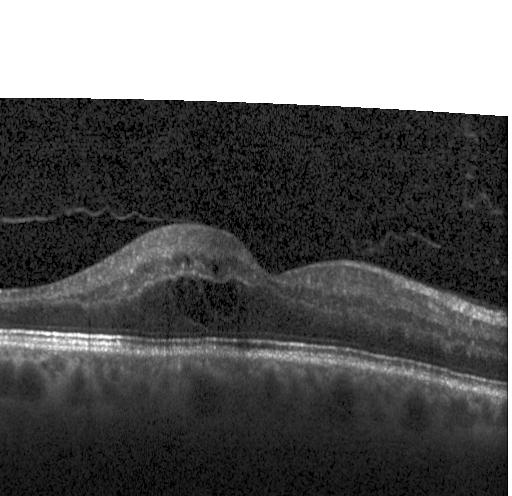

The scan shows DME.